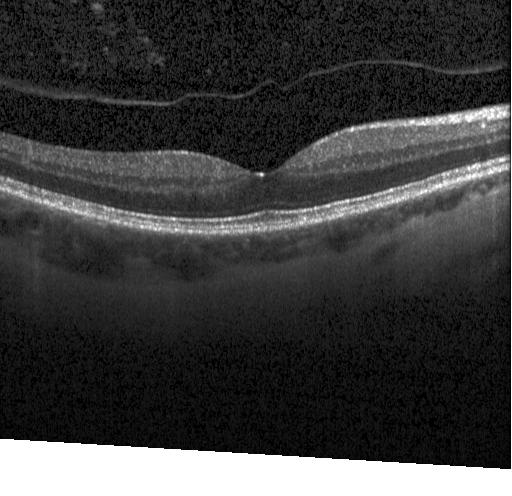

Spectral-domain OCT B-scan: no choroidal neovascularization, diabetic macular edema, or drusen.